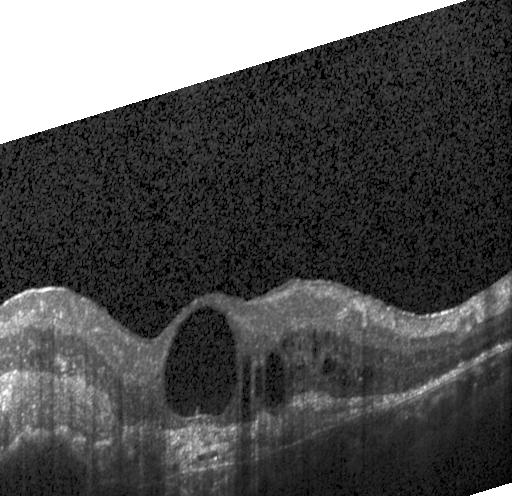 OCT line scan; Heidelberg Spectralis OCT system
Assessment: a choroidal neovascular membrane.